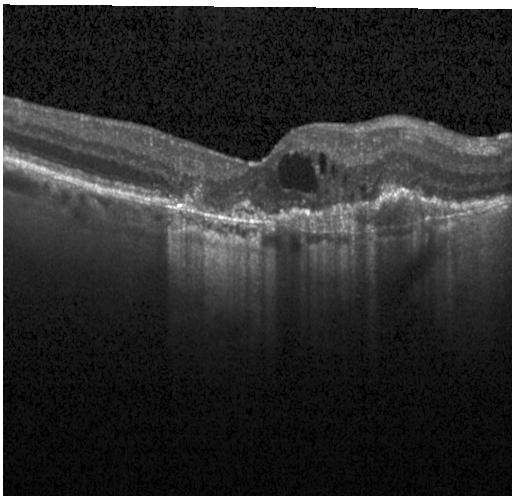
OCT B-scan showing CNV.